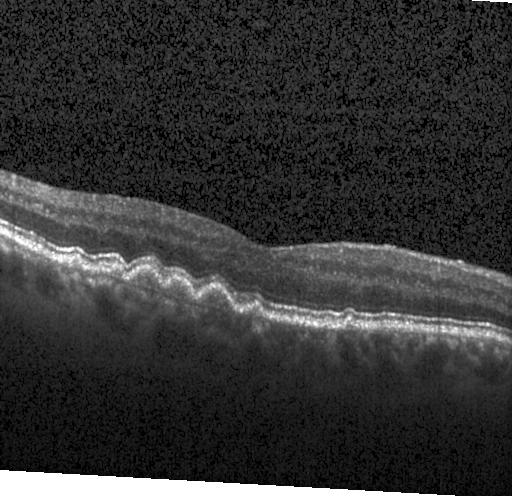

Retinal OCT B-scan. Horizontal scan through the fovea — Impression: drusen.